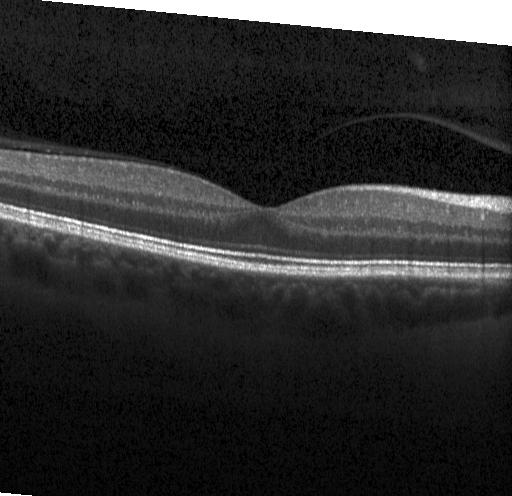

Heidelberg Spectralis. Retinal OCT cross-section
The scan shows neither choroidal neovascularization, diabetic macular edema, nor drusen.